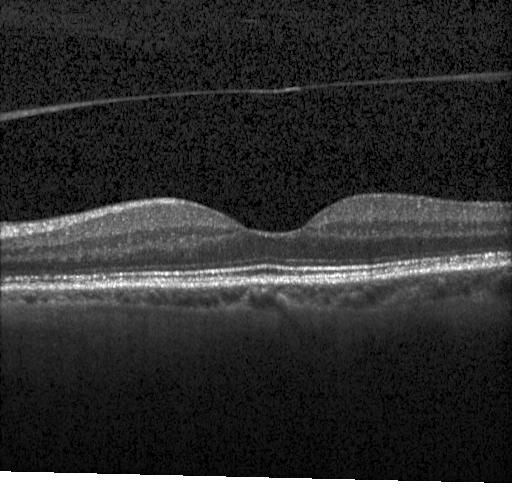

This B-scan demonstrates no choroidal neovascularization, diabetic macular edema, or drusen.